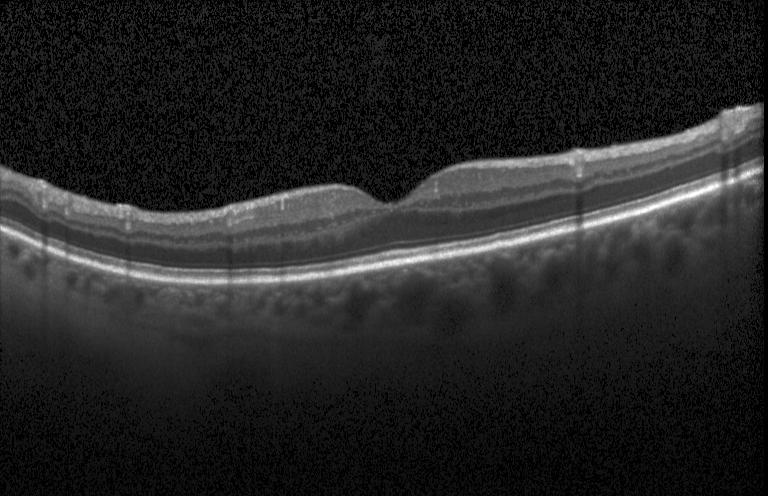
Optical coherence tomography B-scan. Heidelberg Spectralis OCT system. Spectral-domain optical coherence tomography. Macular OCT: no evidence of CNV, DME, or drusen.